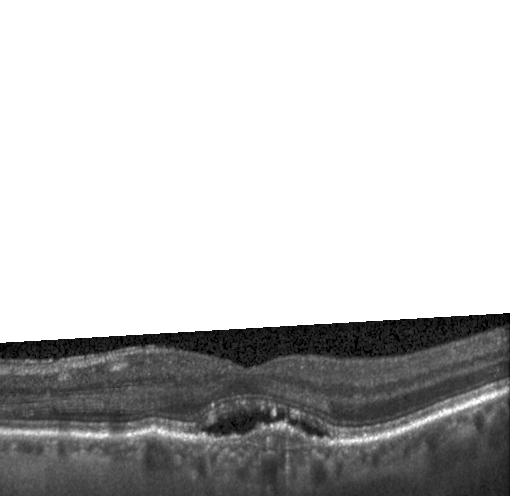

Optical coherence tomography scan — Diagnosis: a choroidal neovascular membrane.